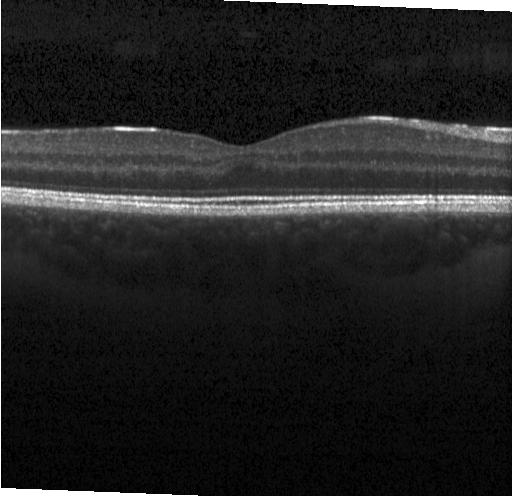 Impression: no CNV, DME, or drusen.